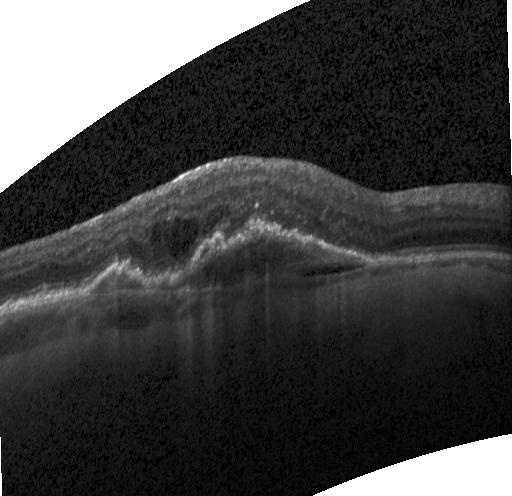
OCT line scan; horizontal scan through the fovea. Finding: a choroidal neovascular membrane.